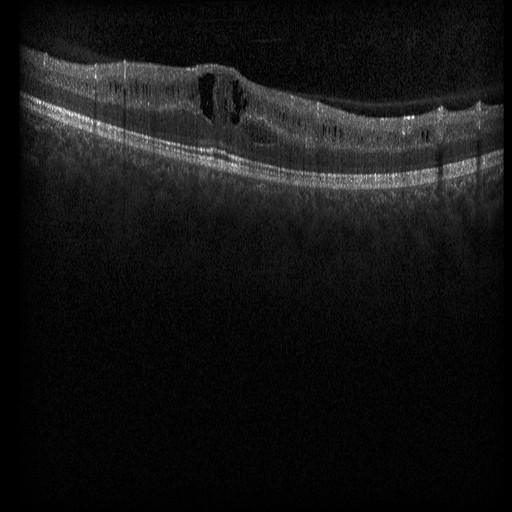

Assessment: diabetic macular edema.